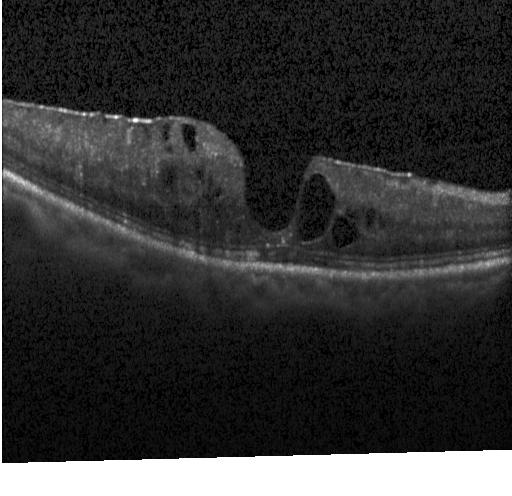

The scan shows diabetic macular edema.